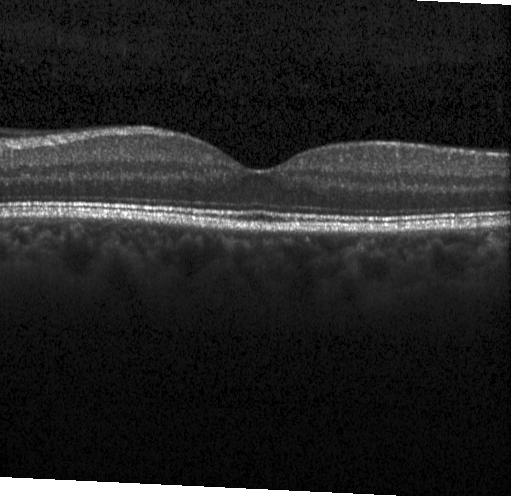
SD-OCT · OCT line scan · macular scan.
Macular OCT: neither choroidal neovascularization, diabetic macular edema, nor drusen.